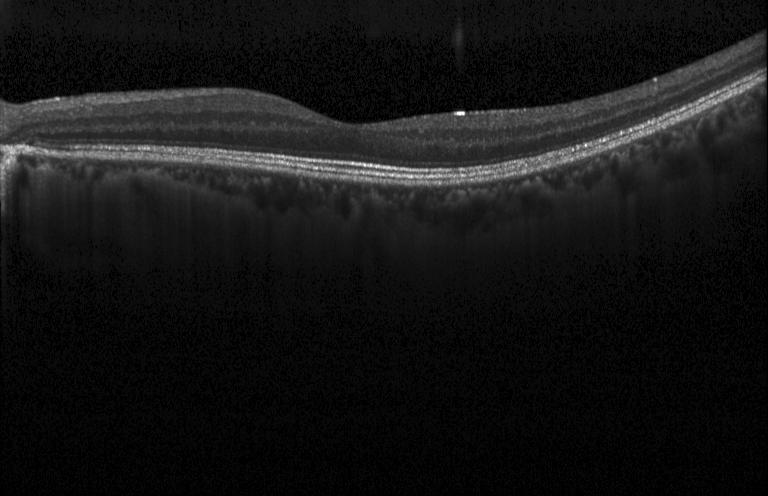

Retinal OCT B-scan.
The scan shows neither CNV, DME, nor drusen.